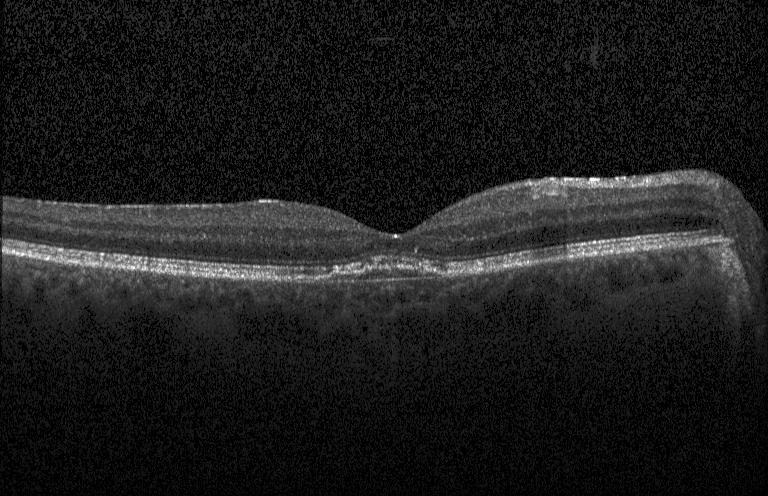 OCT B-scan
A choroidal neovascular membrane.